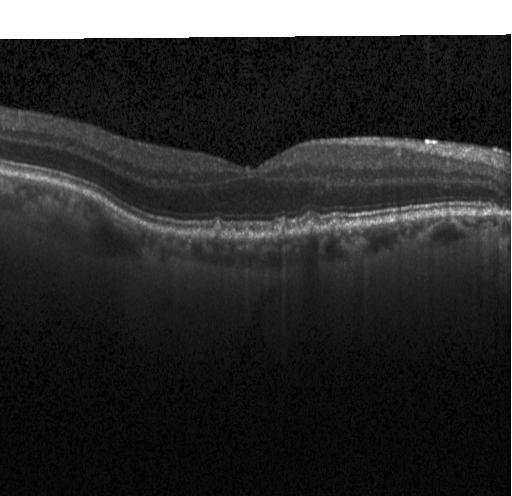
Finding: sub-RPE drusenoid deposits.